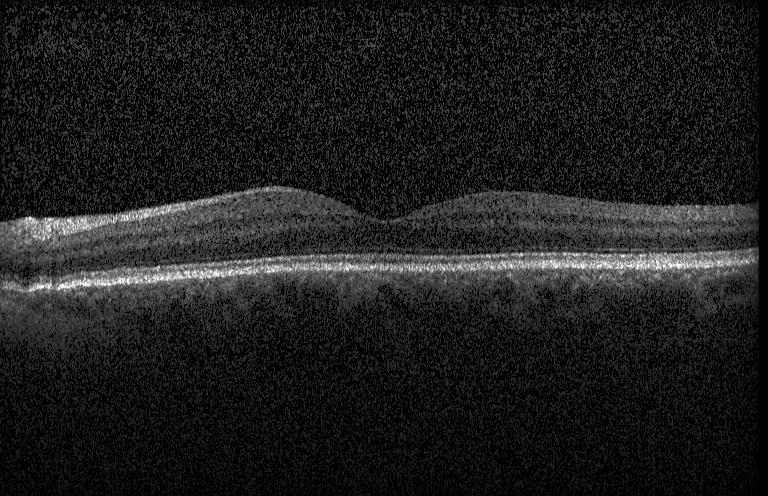
Spectral-domain OCT B-scan: no CNV, DME, or drusen.